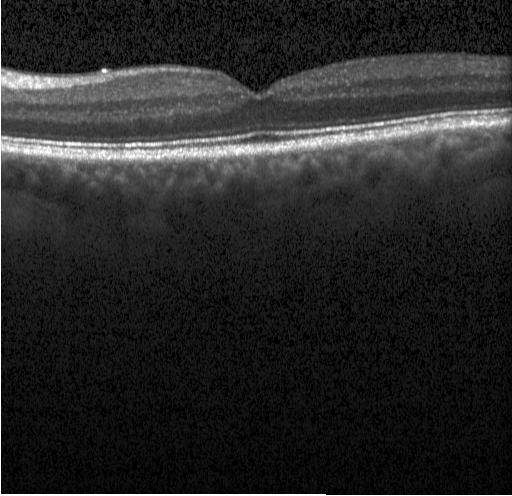
Retinal OCT cross-section — This B-scan demonstrates neither choroidal neovascularization, diabetic macular edema, nor drusen.